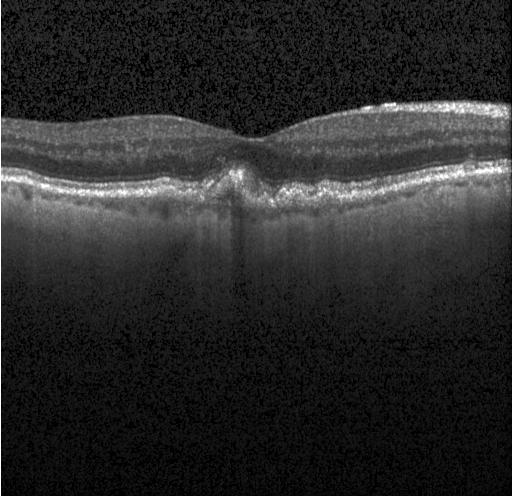 Impression: drusen.